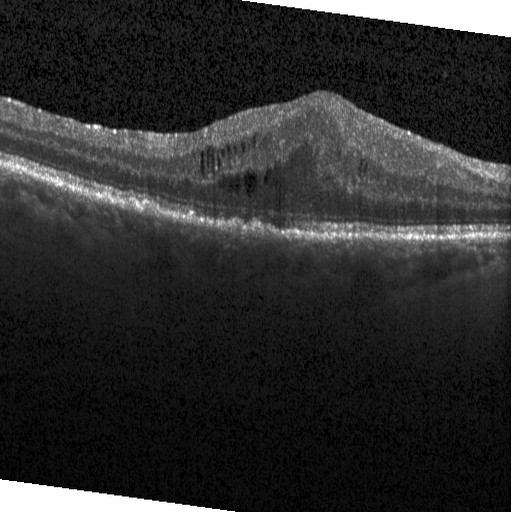

Retinal OCT cross-section showing DME.